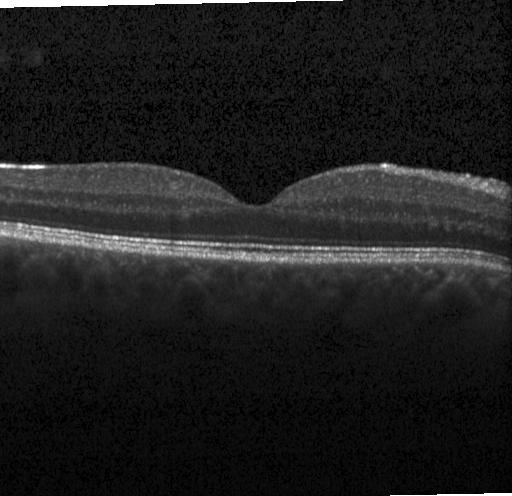
OCT finding: no CNV, DME, or drusen.